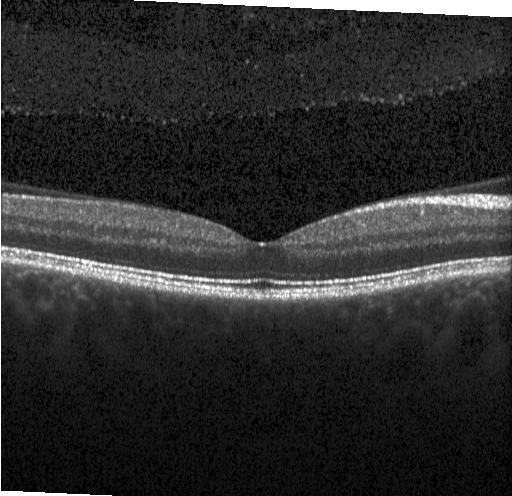
OCT line scan
OCT finding: no choroidal neovascularization, diabetic macular edema, or drusen.